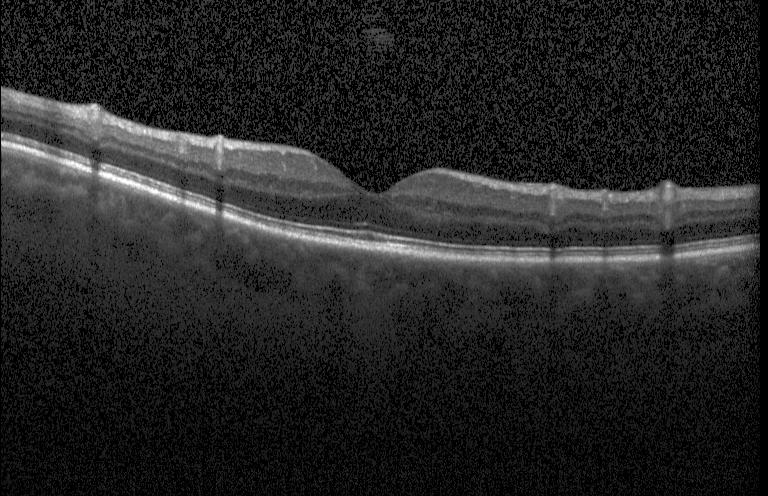
Instrument: Heidelberg Spectralis. Fovea-centered. Retinal OCT cross-section
Diagnosis: no CNV, DME, or drusen.